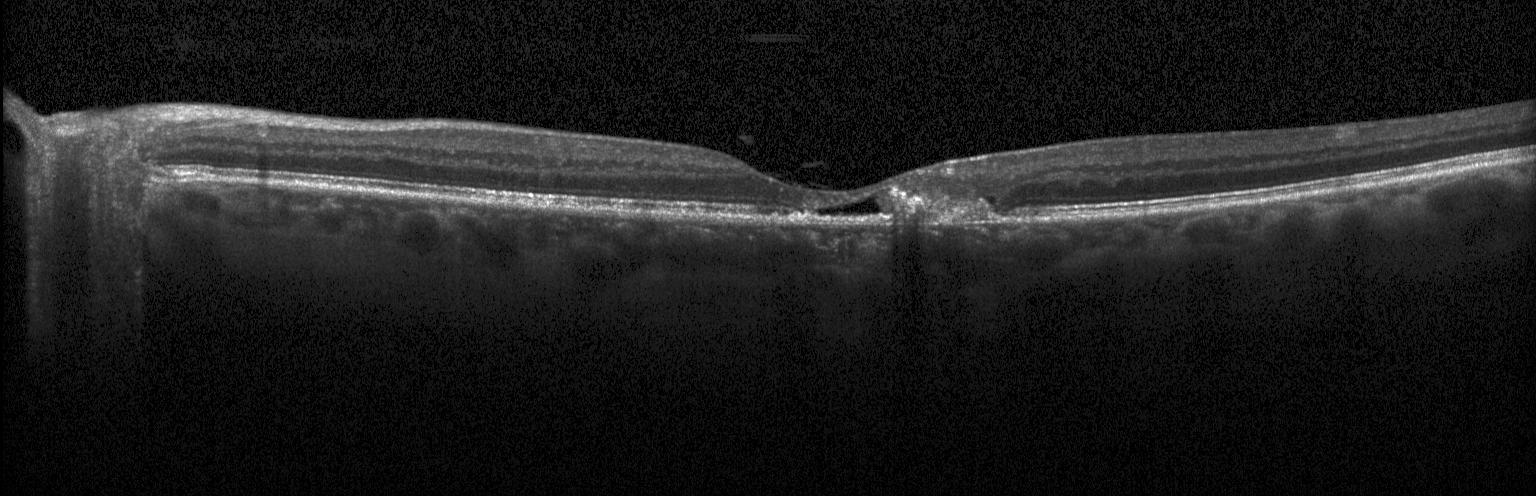

Finding: choroidal neovascularization (CNV).